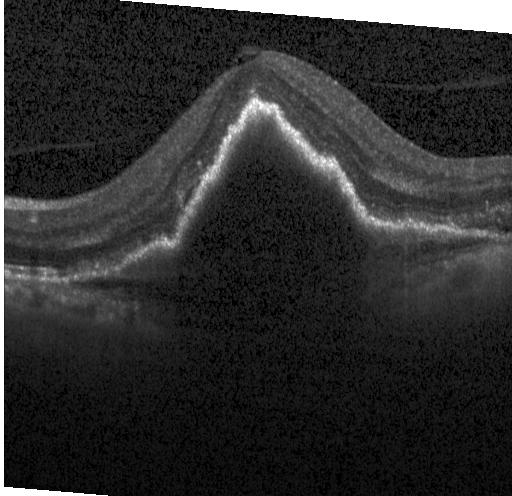

Optical coherence tomography scan · horizontal scan through the fovea. Assessment: a choroidal neovascular membrane.